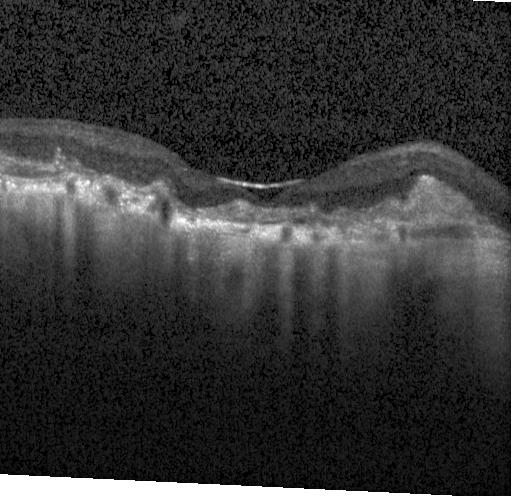

Heidelberg Spectralis OCT system, OCT line scan, spectral-domain optical coherence tomography.
Diagnosis: a choroidal neovascular membrane.